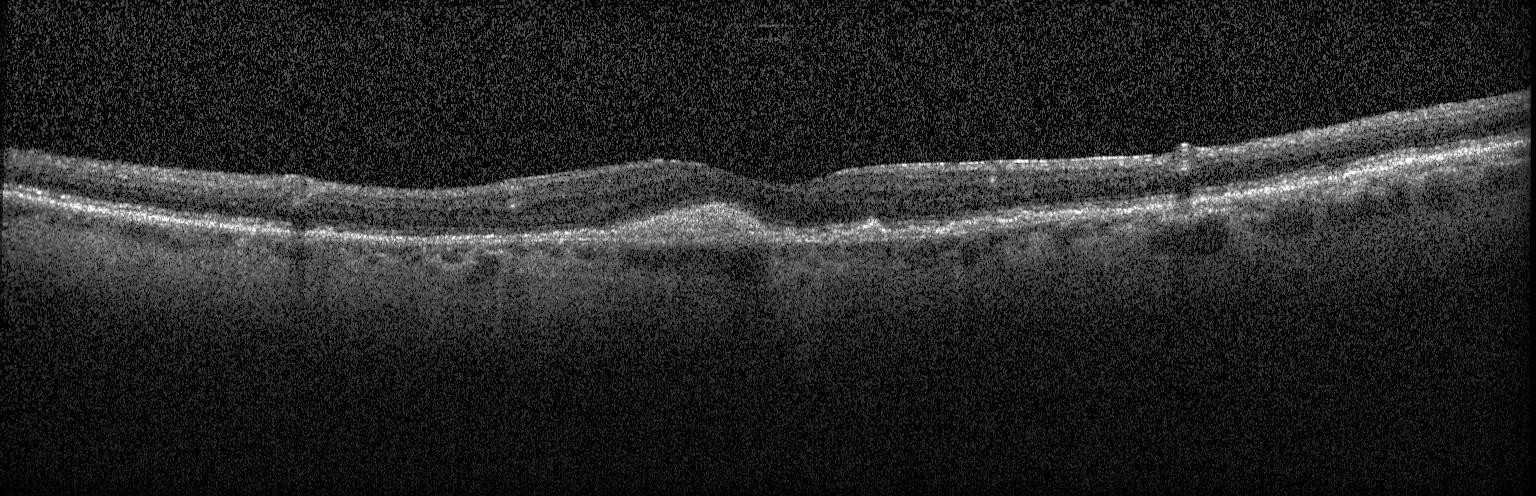
Macular scan. OCT B-scan. Acquired on a Heidelberg Spectralis.
This B-scan demonstrates a choroidal neovascular membrane.